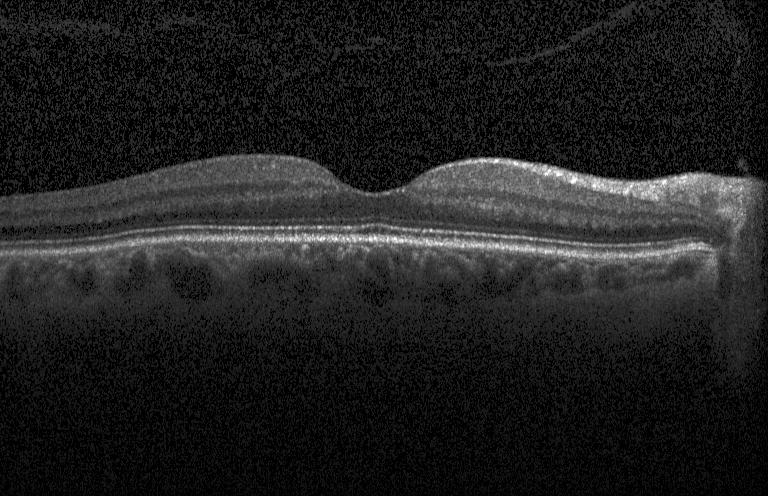 OCT B-scan — Dx: no evidence of CNV, DME, or drusen.